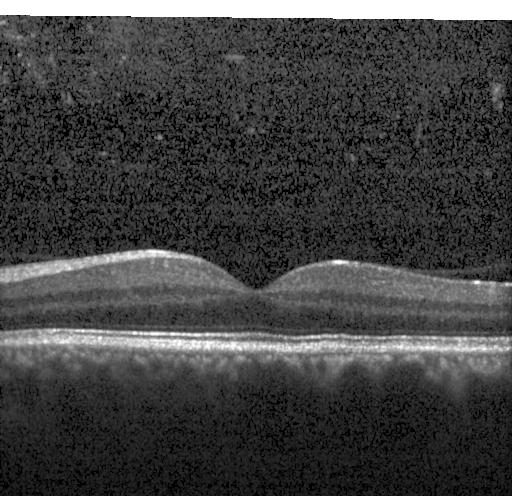

Optical coherence tomography scan; spectral-domain OCT; horizontal scan through the fovea — OCT finding: no CNV, no DME, and no drusen.